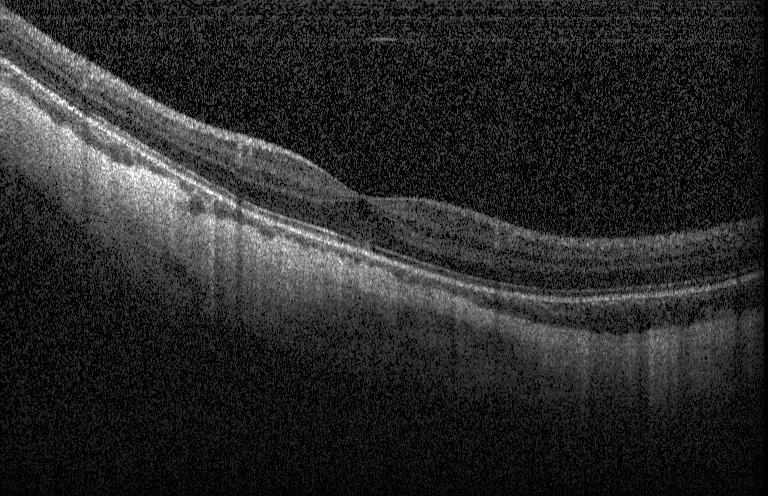
Spectral-domain OCT B-scan: diabetic macular edema (DME).